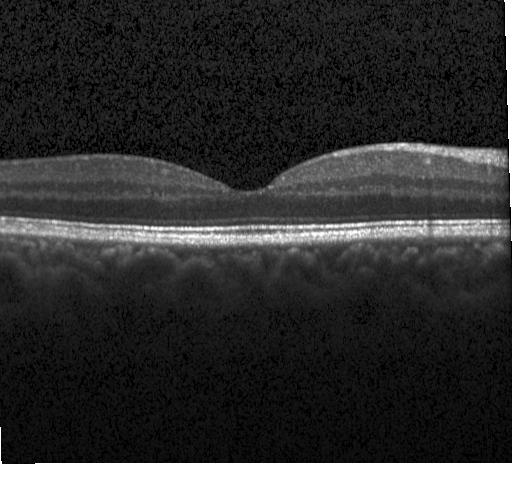
Fovea-centered, retinal OCT B-scan.
Impression: no choroidal neovascularization, no diabetic macular edema, and no drusen.